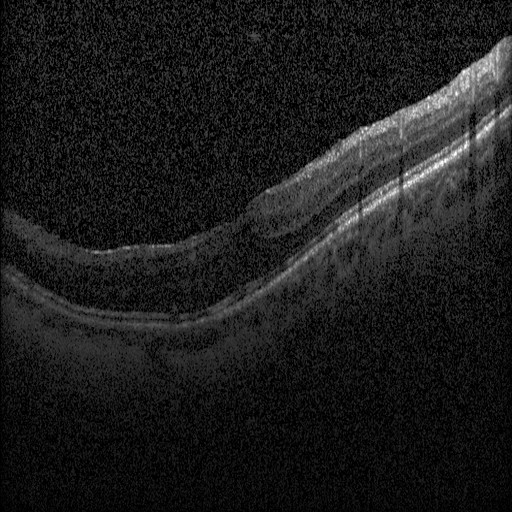 Retinal OCT B-scan. Impression: diabetic macular edema.